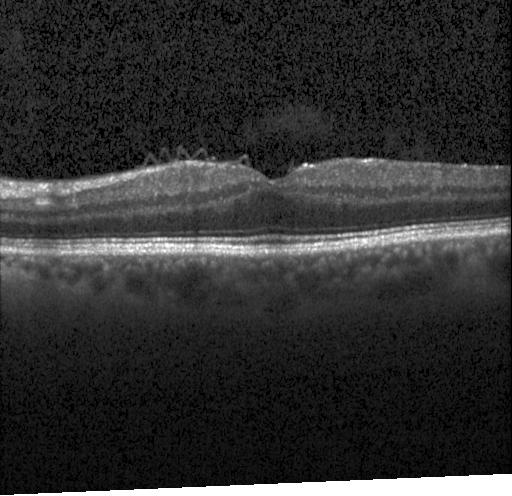 OCT B-scan — Macular OCT: no evidence of CNV, DME, or drusen.